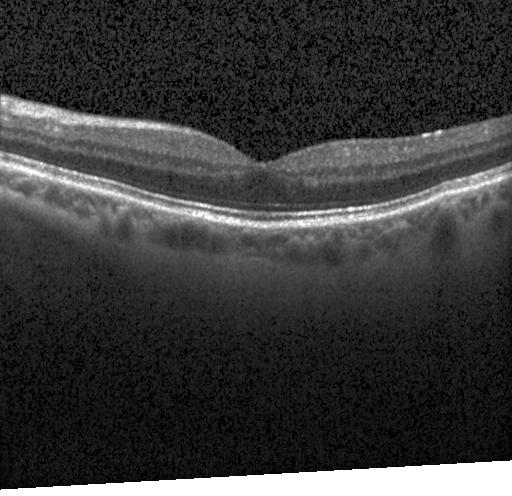
Diagnosis: no choroidal neovascularization, no diabetic macular edema, and no drusen.